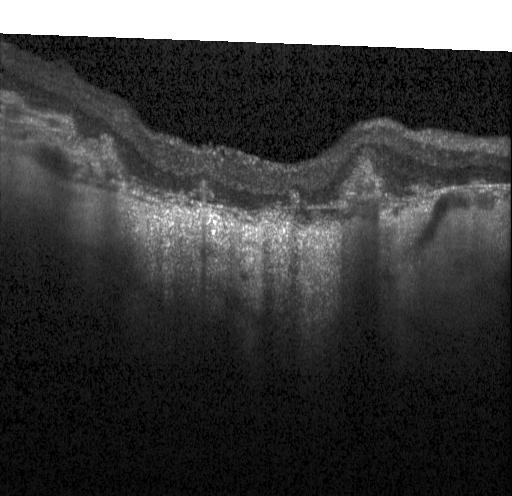

OCT line scan. Diagnosis: choroidal neovascularization (CNV).